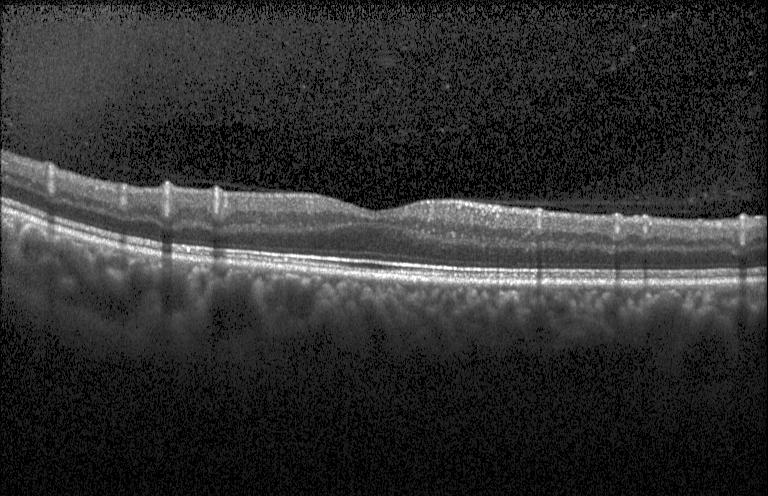 Optical coherence tomography B-scan; centered on the fovea; acquired on a Heidelberg Spectralis — Dx: no CNV, DME, or drusen.